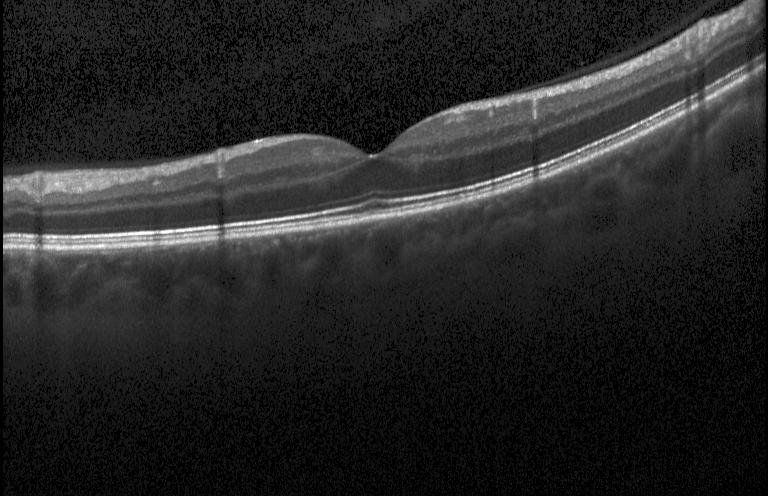

Impression: no choroidal neovascularization, diabetic macular edema, or drusen.